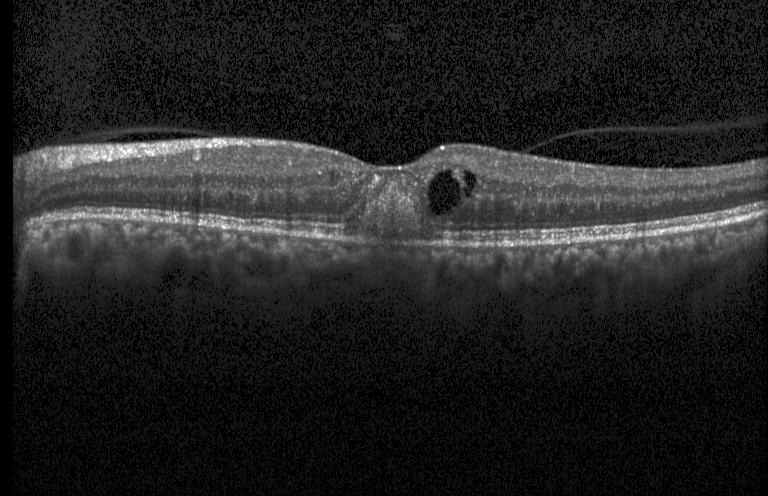 Finding: a choroidal neovascular membrane.